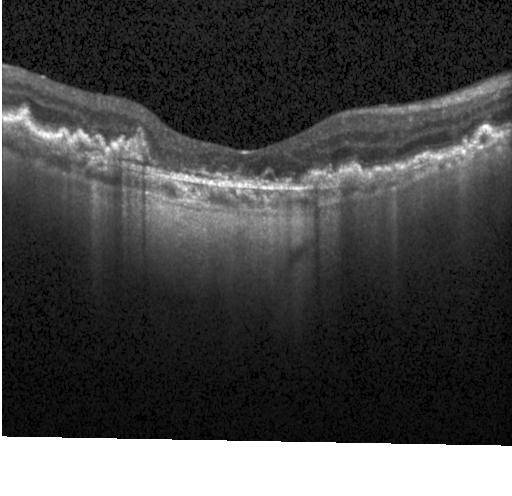

Spectral-domain OCT B-scan: CNV.